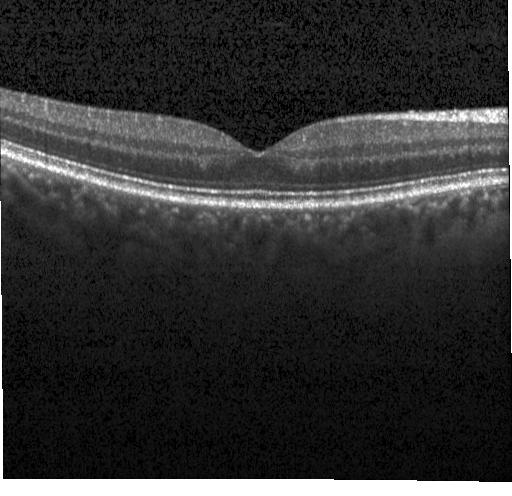
OCT B-scan — Diagnosis: no evidence of choroidal neovascularization, diabetic macular edema, or drusen.